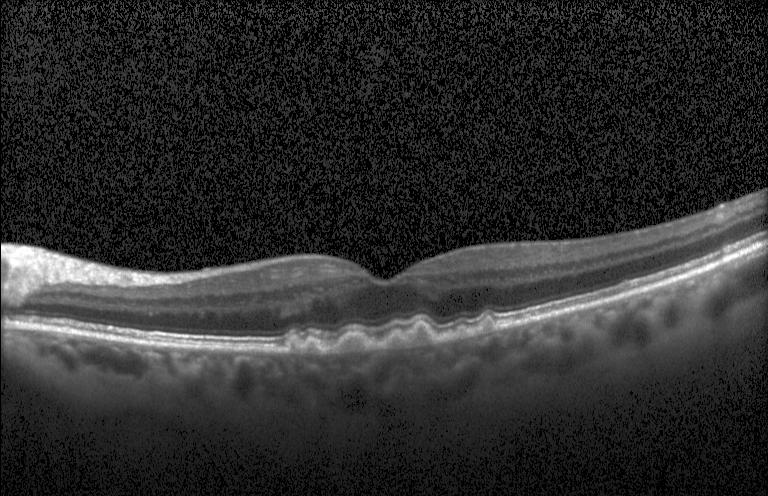

OCT B-scan showing multiple drusen.